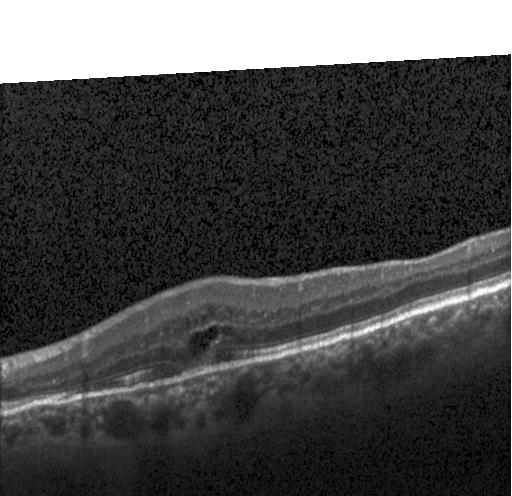
OCT line scan. Finding: DME.